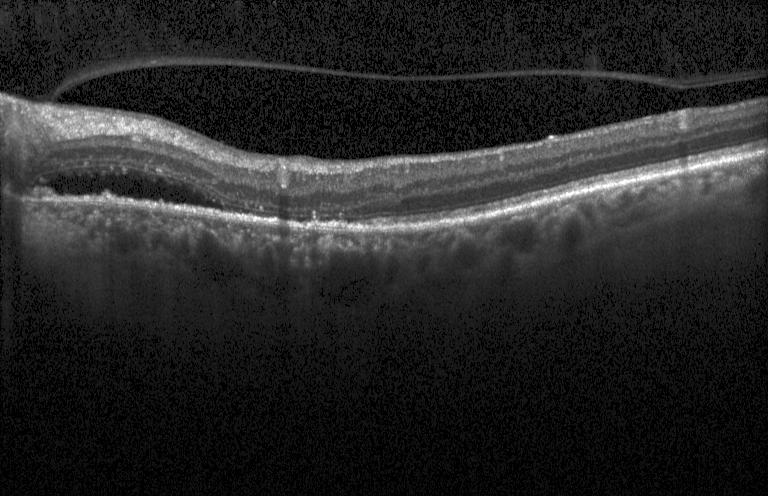 Macular scan, spectral-domain OCT, OCT B-scan. This B-scan demonstrates a choroidal neovascular membrane.